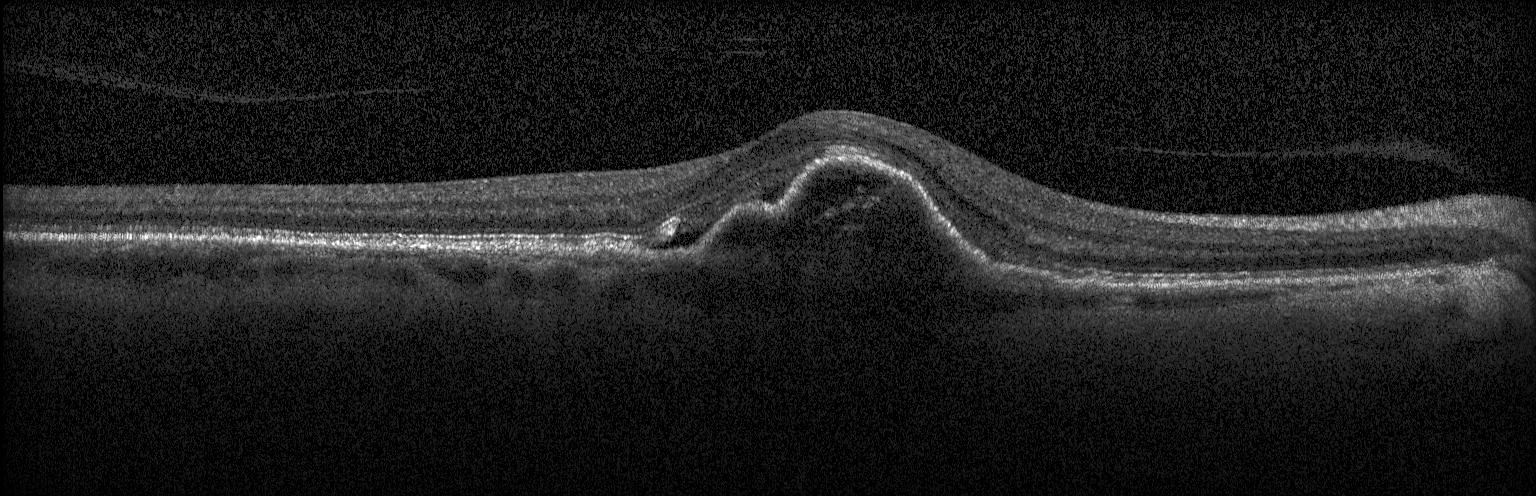 Through the macula; optical coherence tomography B-scan; Heidelberg Spectralis; spectral-domain OCT
Finding: a choroidal neovascular membrane.